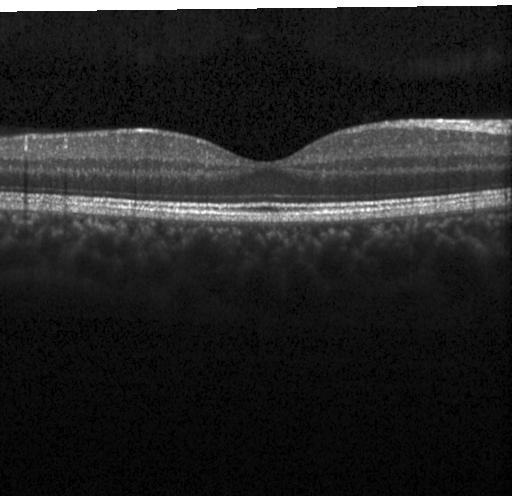 OCT B-scan showing no evidence of choroidal neovascularization, diabetic macular edema, or drusen.